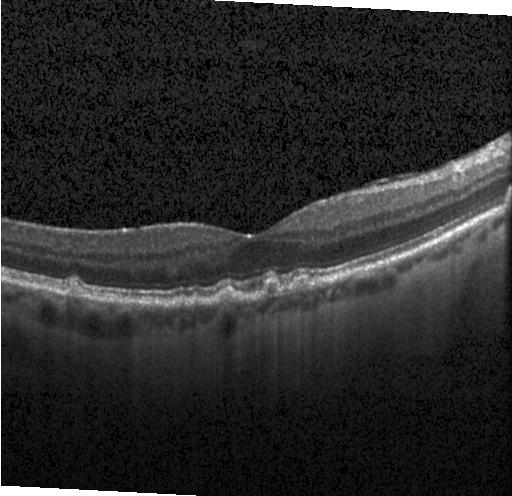
Spectral-domain optical coherence tomography · instrument: Heidelberg Spectralis · retinal OCT B-scan — Diagnosis: sub-RPE drusenoid deposits.